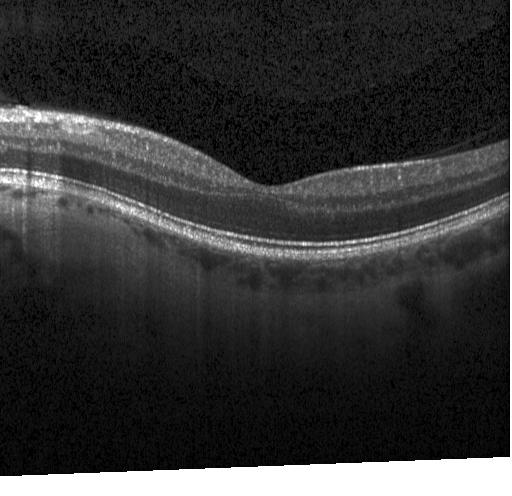 Diagnosis: no choroidal neovascularization, diabetic macular edema, or drusen.